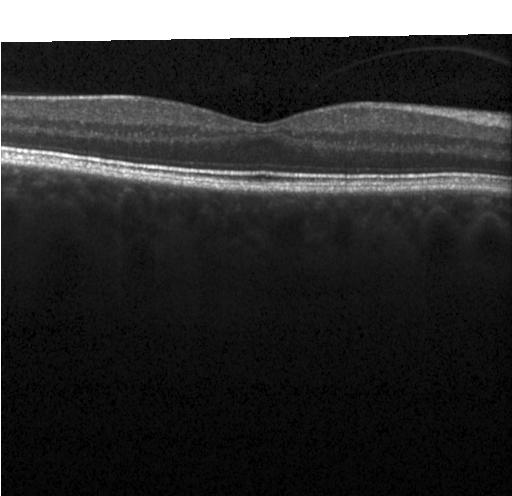
OCT finding: no choroidal neovascularization, diabetic macular edema, or drusen.